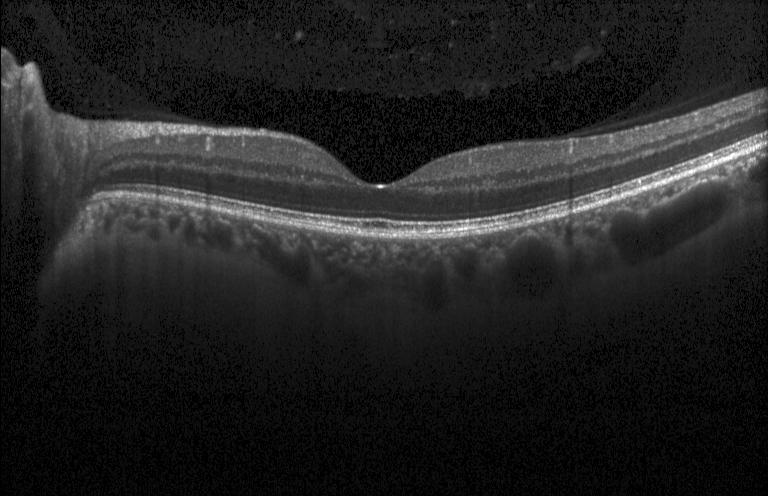 Spectral-domain OCT; optical coherence tomography B-scan; acquired on a Heidelberg Spectralis
Impression: no evidence of CNV, DME, or drusen.